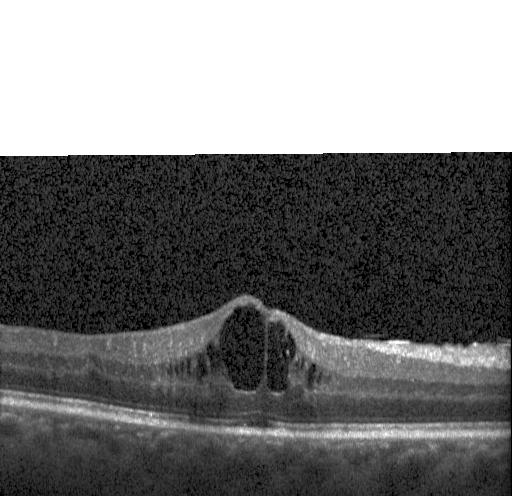 Assessment: diabetic macular edema.